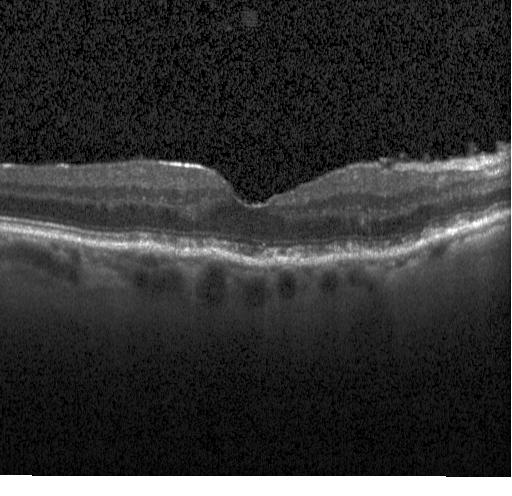
Diagnosis: multiple drusen.